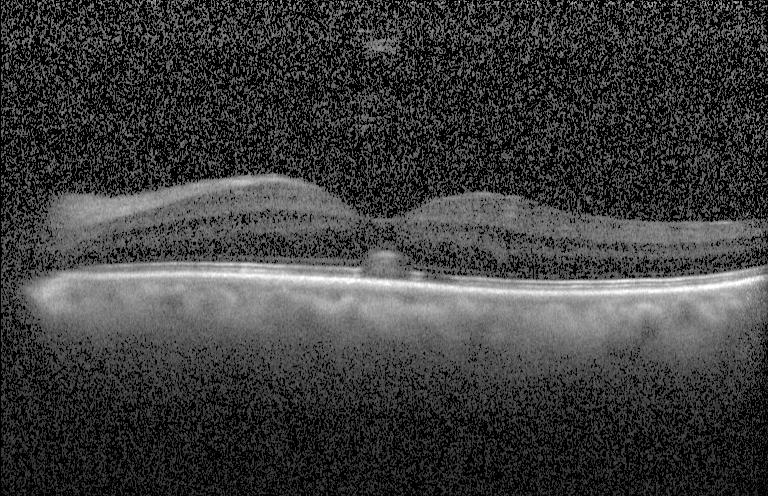
Dx: choroidal neovascularization (CNV).